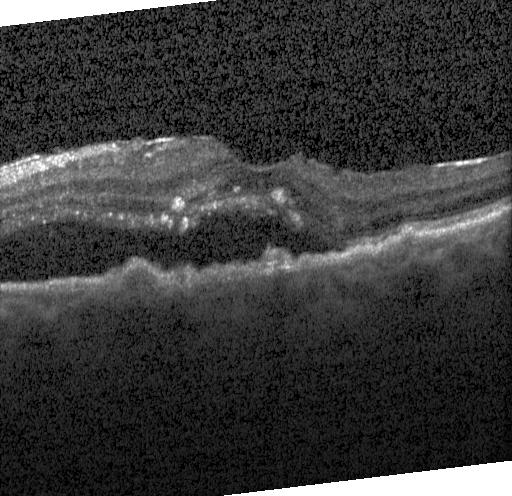 Instrument: Heidelberg Spectralis · optical coherence tomography B-scan · through the macula — This B-scan demonstrates a choroidal neovascular membrane.